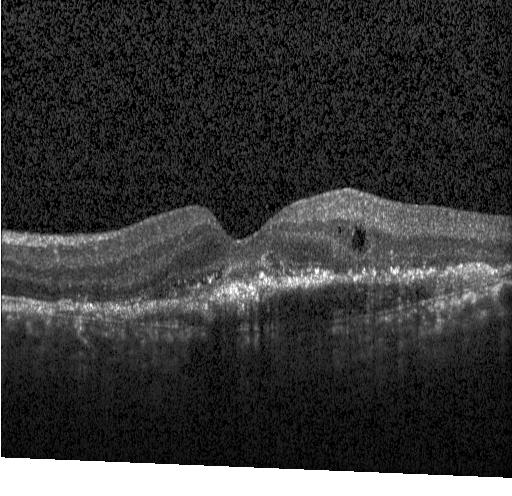 Retinal OCT B-scan. Heidelberg Spectralis OCT system.
Finding: choroidal neovascularization (CNV).